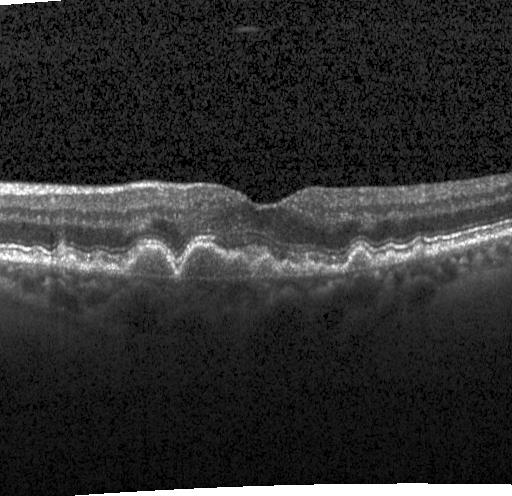 The scan shows a choroidal neovascular membrane.